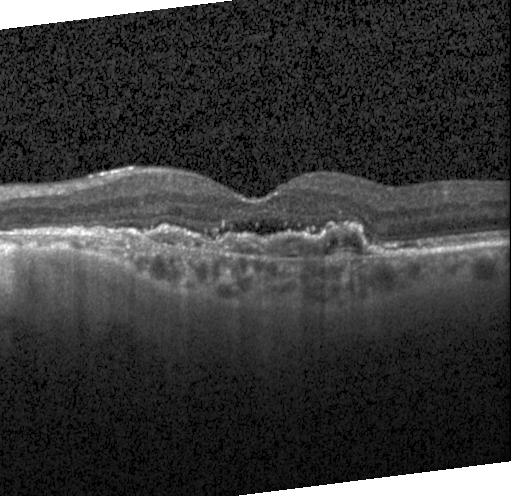 Diagnosis: choroidal neovascularization (CNV).